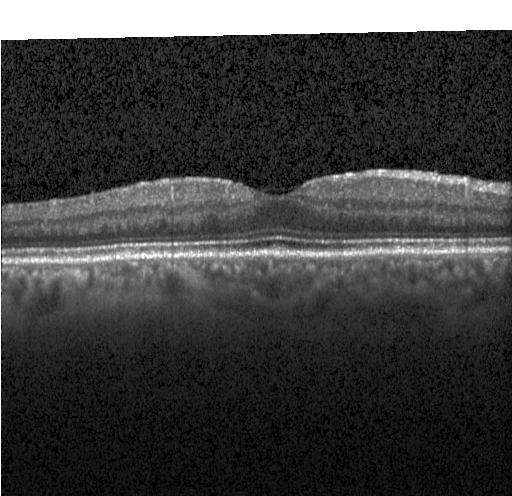

SD-OCT · instrument: Heidelberg Spectralis · horizontal scan through the fovea · optical coherence tomography scan.
Diagnosis: no choroidal neovascularization, no diabetic macular edema, and no drusen.